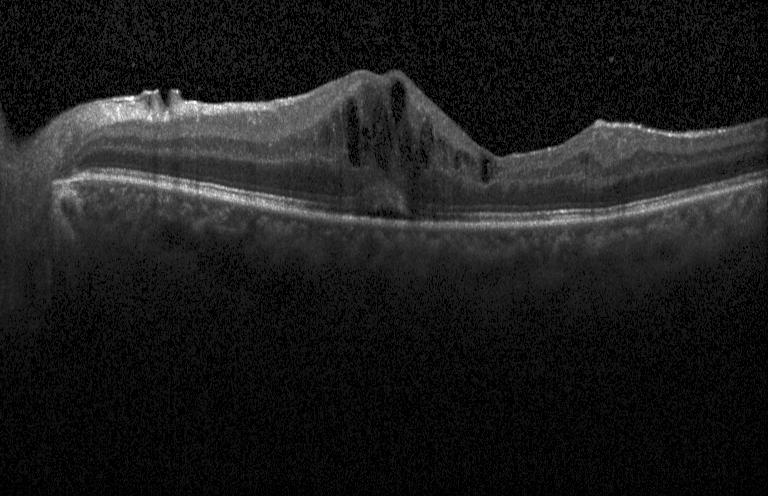 Spectral-domain optical coherence tomography. Optical coherence tomography scan. Instrument: Heidelberg Spectralis. Centered on the fovea — Finding: diabetic macular edema (DME).